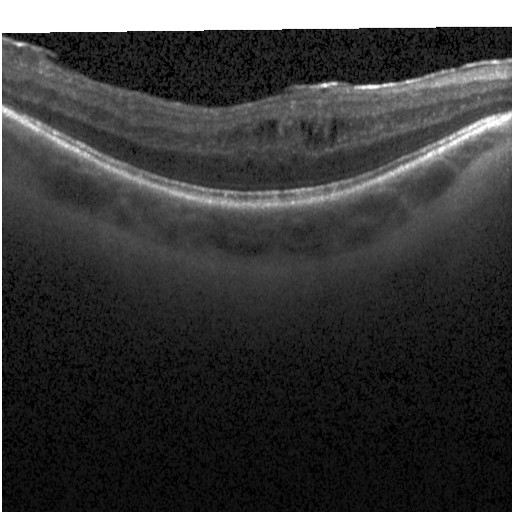
Retinal OCT B-scan — OCT finding: diabetic macular edema (DME).